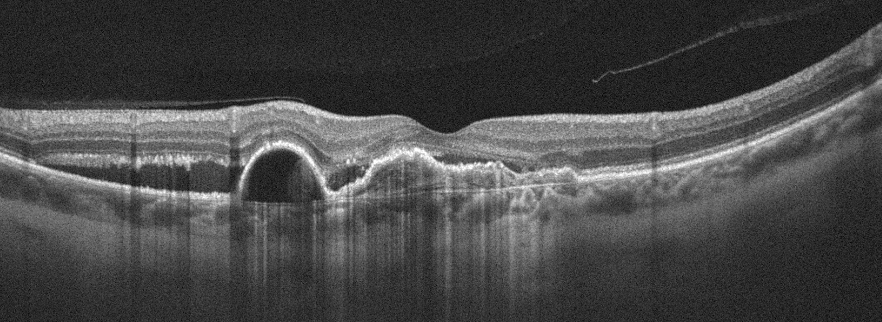 Acquired on an Optovue Avanti RTVue XR, retinal OCT cross-section
Finding: age-related macular degeneration (AMD).